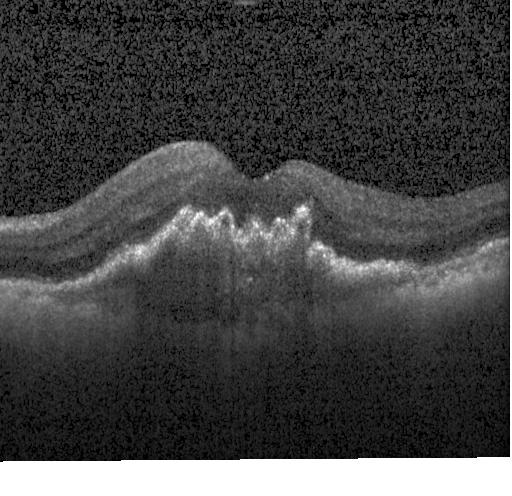

Macular OCT demonstrating a choroidal neovascular membrane.